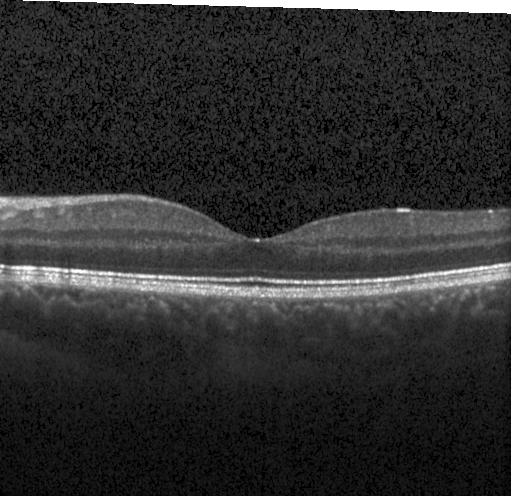

Retinal OCT B-scan. Heidelberg Spectralis OCT system. Impression: no evidence of CNV, DME, or drusen.